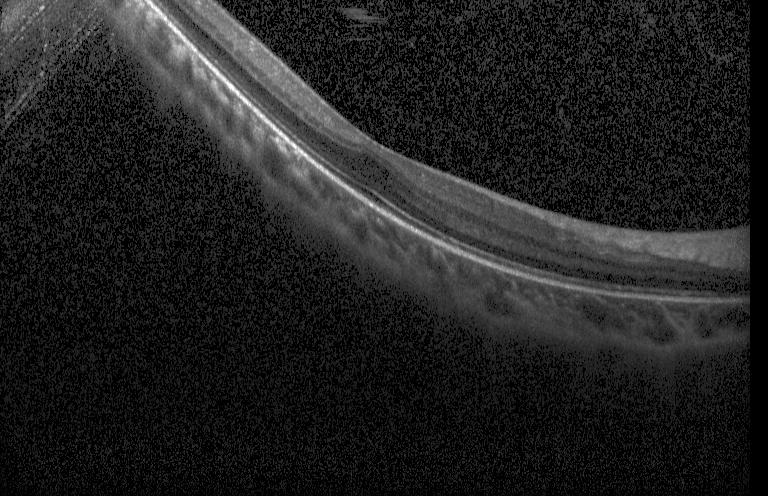
Diagnosis: no choroidal neovascularization, no diabetic macular edema, and no drusen.